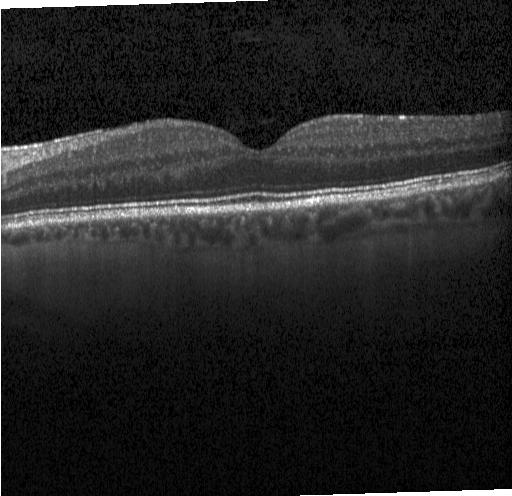

Spectral-domain OCT B-scan: no choroidal neovascularization, diabetic macular edema, or drusen.